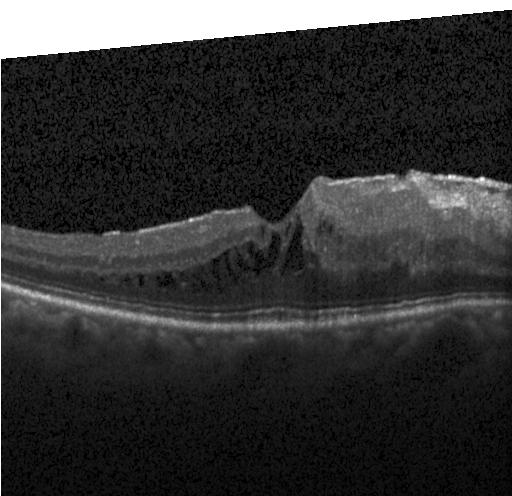

Instrument: Heidelberg Spectralis · spectral-domain optical coherence tomography · macular scan · OCT B-scan.
Finding: diabetic macular edema.